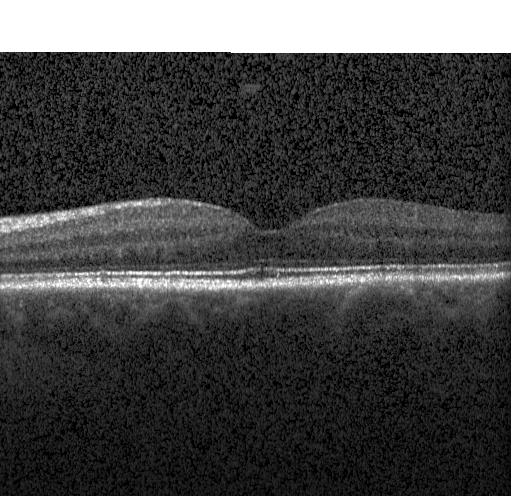 Centered on the fovea, retinal OCT B-scan, acquired on a Heidelberg Spectralis, spectral-domain OCT — Macular OCT: no CNV, DME, or drusen.